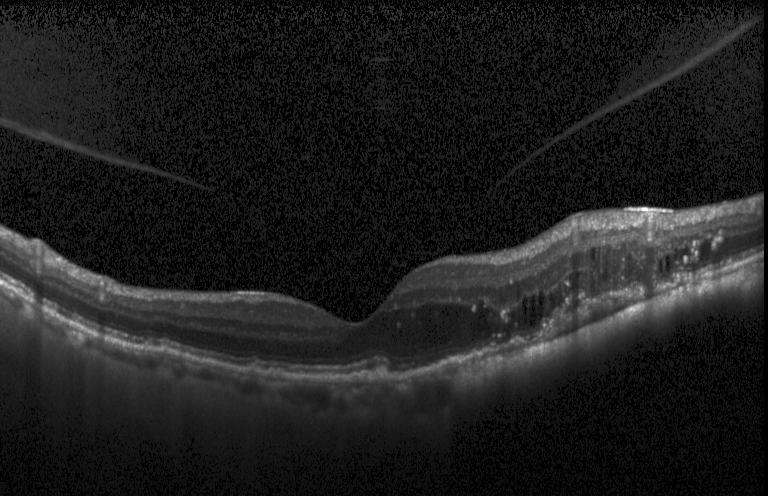
Impression: CNV.